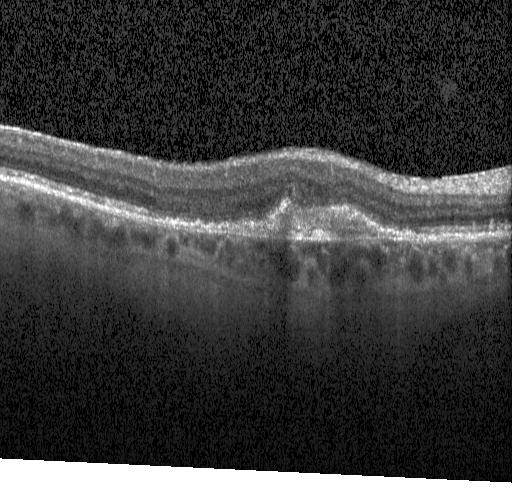

Dx: a choroidal neovascular membrane.